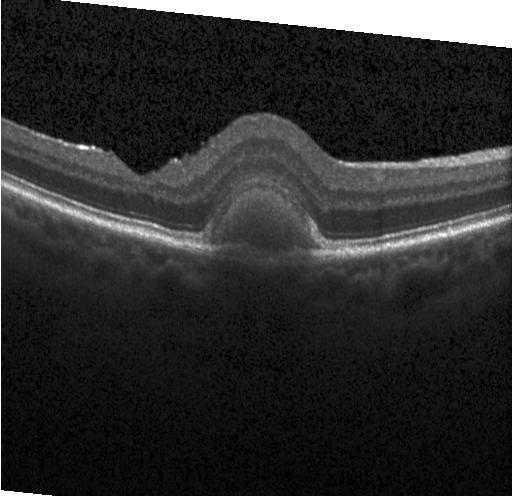 Macular OCT demonstrating CNV.